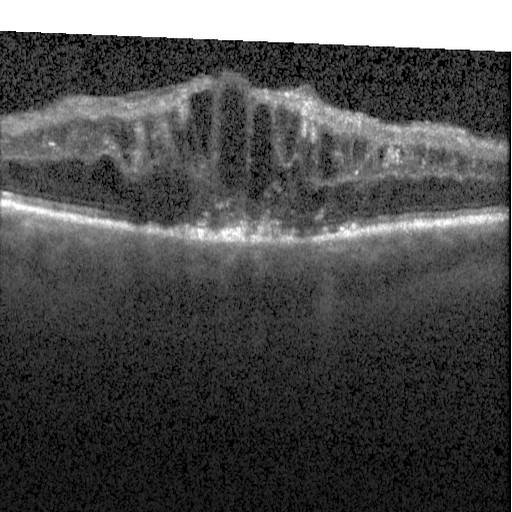
Spectral-domain OCT, retinal OCT cross-section, Heidelberg Spectralis, horizontal scan through the fovea. Impression: diabetic macular edema.